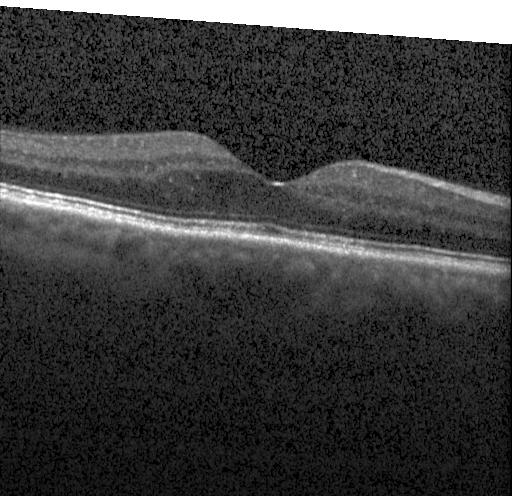 Assessment: no evidence of choroidal neovascularization, diabetic macular edema, or drusen.